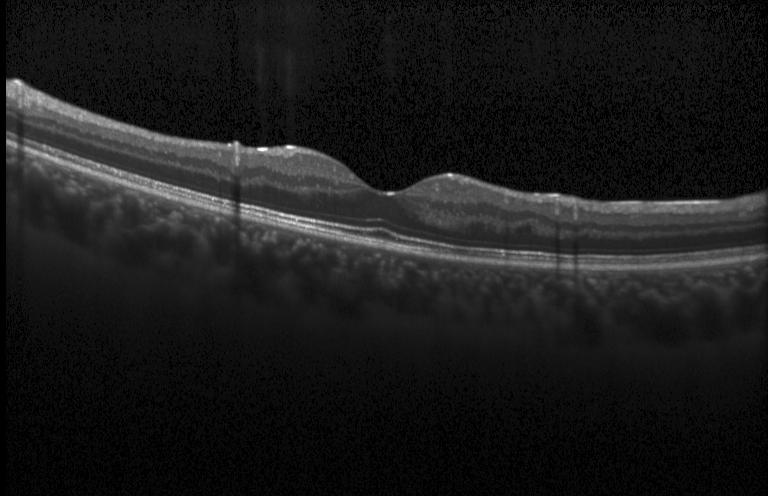
OCT finding: neither CNV, DME, nor drusen.